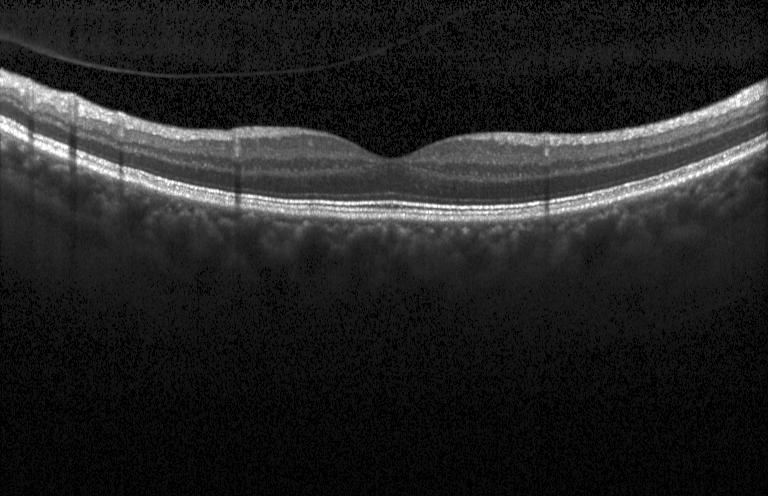
The scan shows no choroidal neovascularization, no diabetic macular edema, and no drusen.